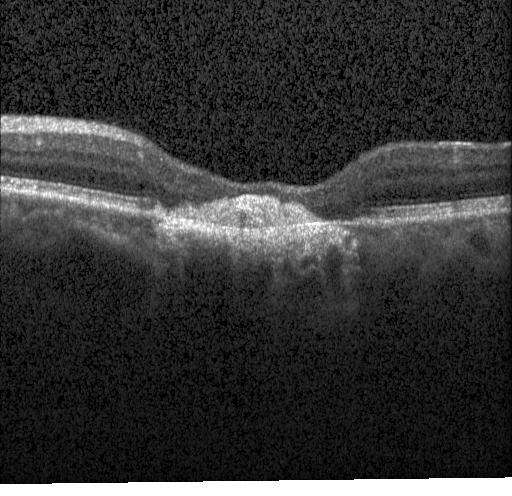 OCT line scan · instrument: Heidelberg Spectralis — Diagnosis: choroidal neovascularization (CNV).